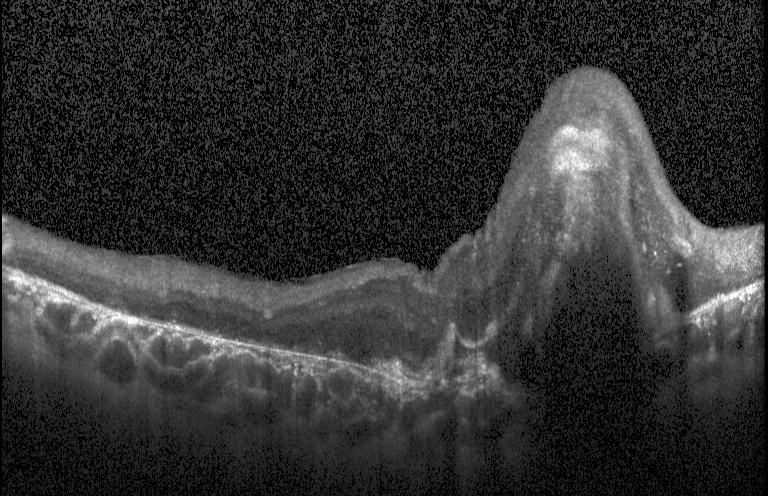

Assessment: CNV.